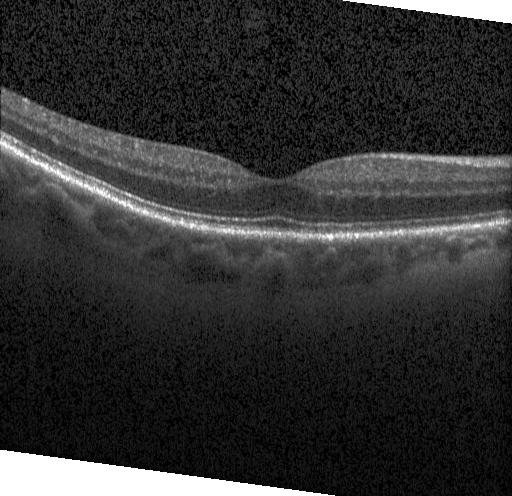

Heidelberg Spectralis; SD-OCT; OCT line scan; horizontal scan through the fovea
Assessment: neither choroidal neovascularization, diabetic macular edema, nor drusen.